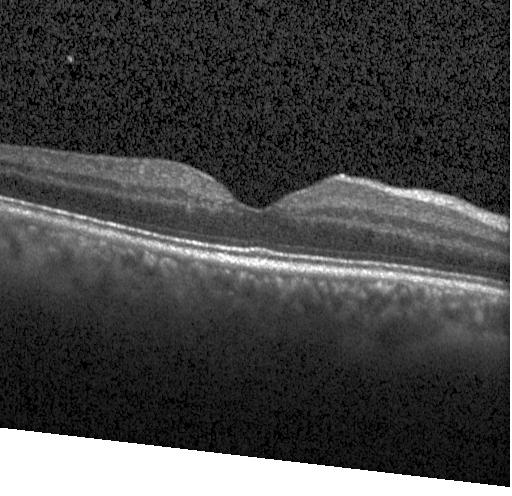
OCT B-scan — Assessment: no choroidal neovascularization, diabetic macular edema, or drusen.